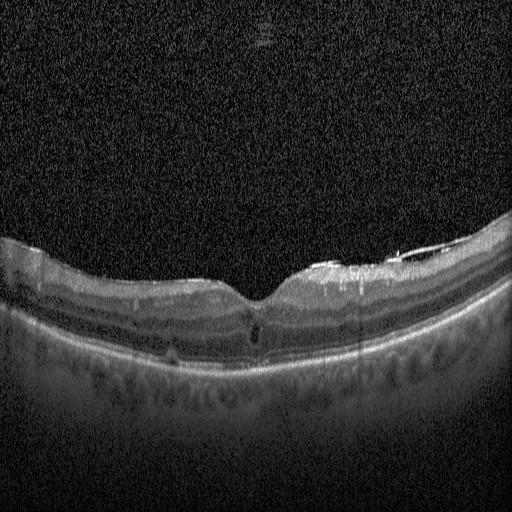

Retinal OCT B-scan.
OCT finding: diabetic macular edema (DME).